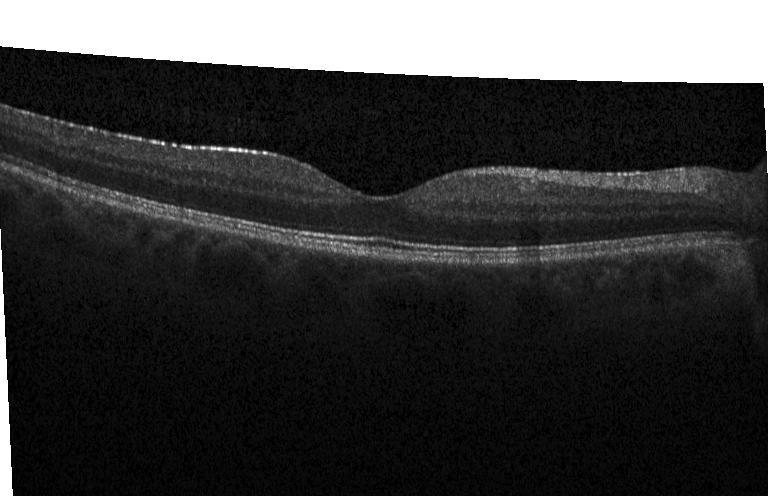

Retinal OCT B-scan, horizontal scan through the fovea
The scan shows neither CNV, DME, nor drusen.